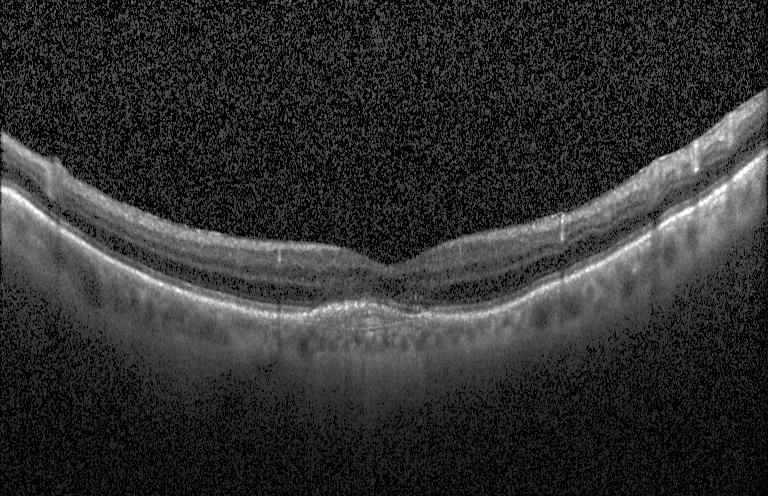

OCT B-scan · horizontal scan through the fovea · SD-OCT — Impression: a choroidal neovascular membrane.